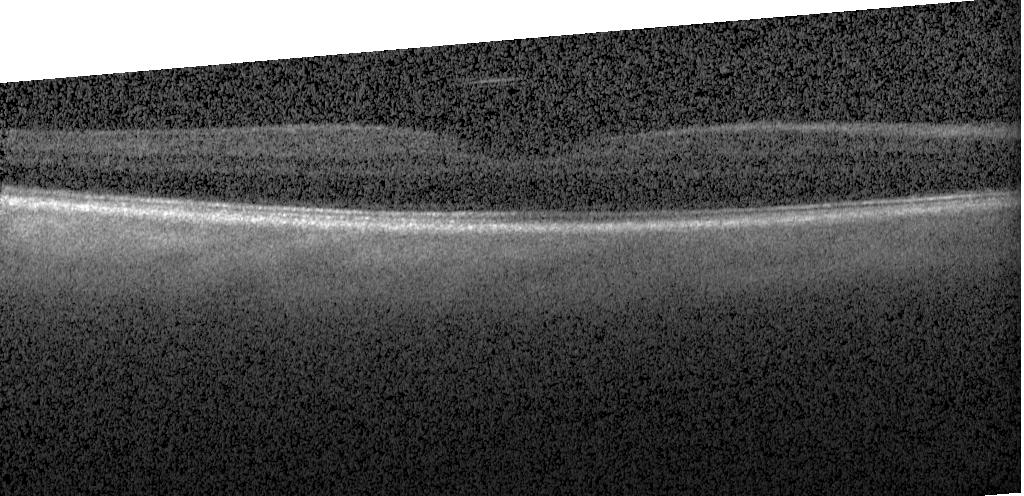

Fovea-centered. OCT line scan.
Diagnosis: no choroidal neovascularization, no diabetic macular edema, and no drusen.